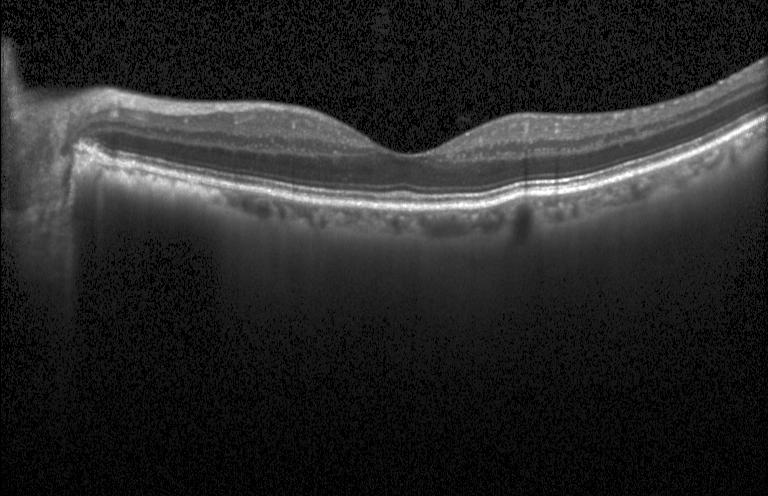

Acquired on a Heidelberg Spectralis; centered on the fovea; SD-OCT; retinal OCT cross-section. Impression: no choroidal neovascularization, diabetic macular edema, or drusen.